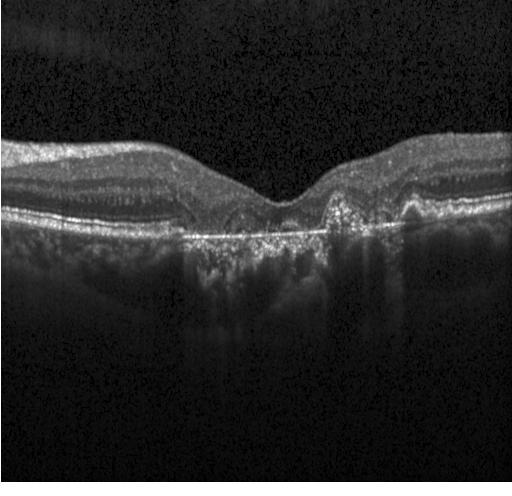

Spectral-domain optical coherence tomography · OCT line scan · macular scan
Choroidal neovascularization (CNV).